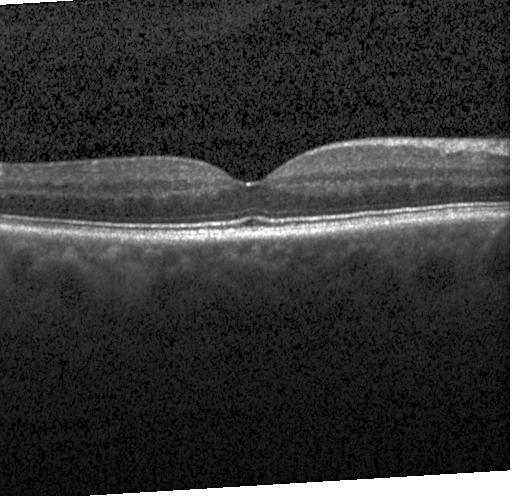

Acquired on a Heidelberg Spectralis · OCT B-scan
Impression: neither choroidal neovascularization, diabetic macular edema, nor drusen.